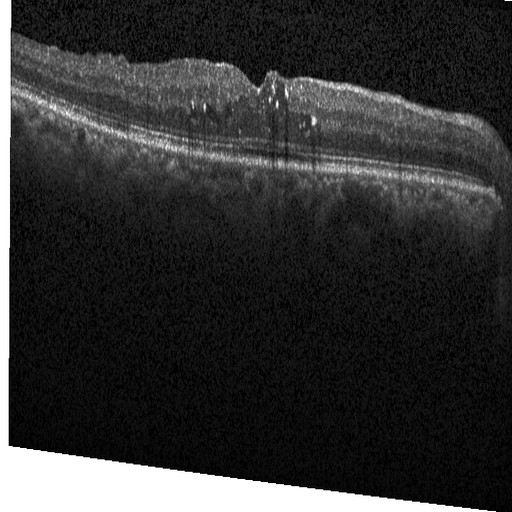 Spectral-domain OCT. Retinal OCT cross-section. Acquired on a Heidelberg Spectralis. Centered on the fovea
Finding: diabetic macular edema.